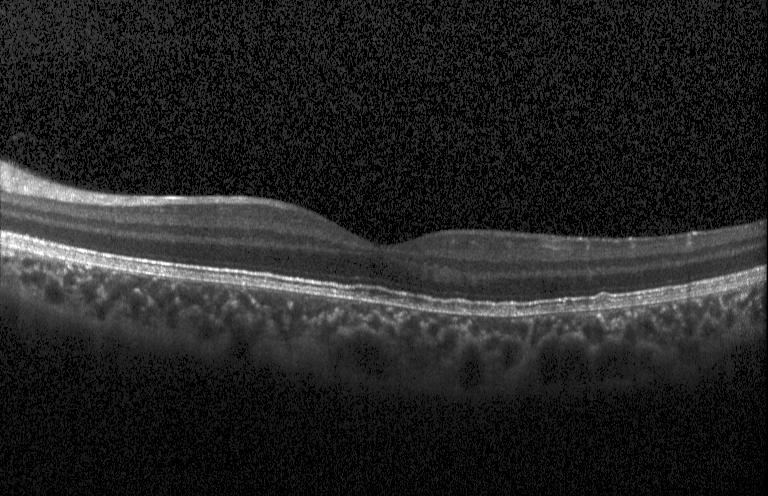
Retinal OCT cross-section, centered on the fovea — This B-scan demonstrates neither choroidal neovascularization, diabetic macular edema, nor drusen.